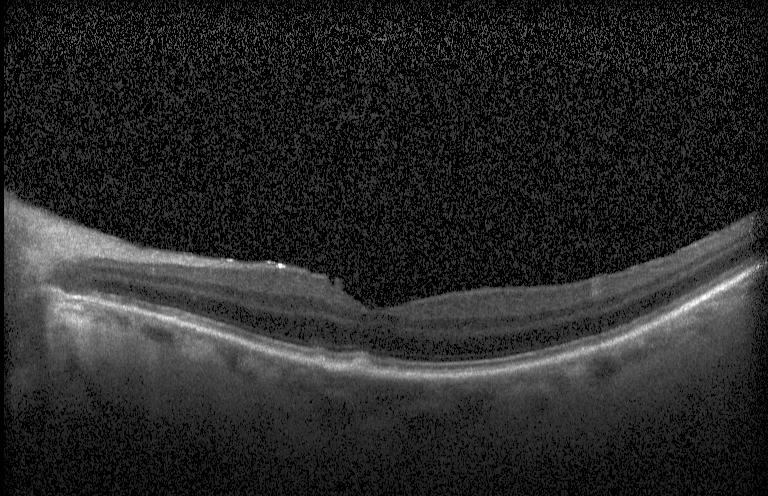

Optical coherence tomography B-scan.
OCT finding: sub-RPE drusenoid deposits.